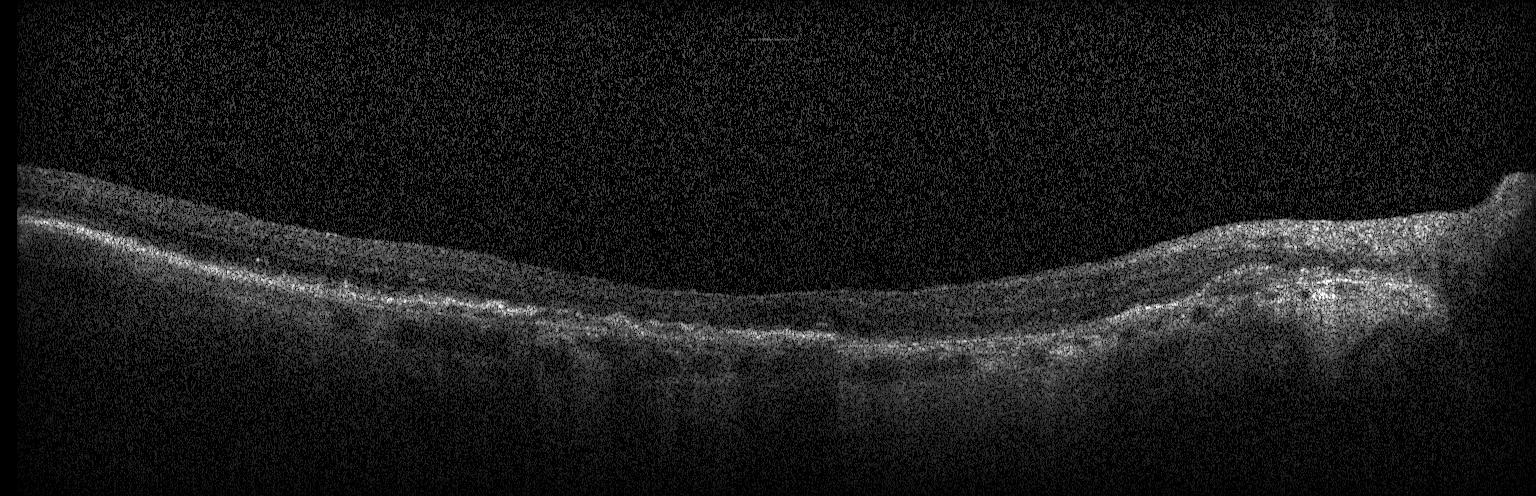
Retinal OCT B-scan. Diagnosis: a choroidal neovascular membrane.